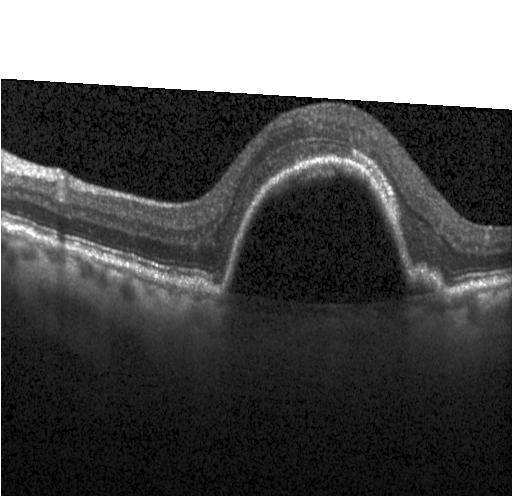 Dx: a choroidal neovascular membrane.